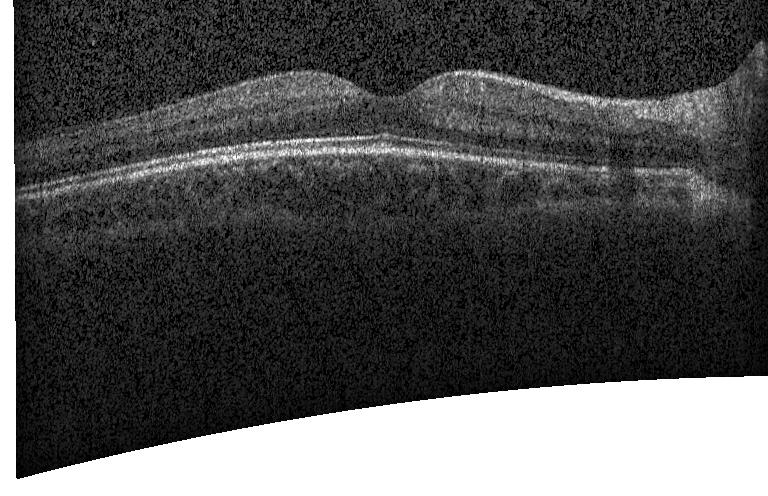

The scan shows neither choroidal neovascularization, diabetic macular edema, nor drusen.